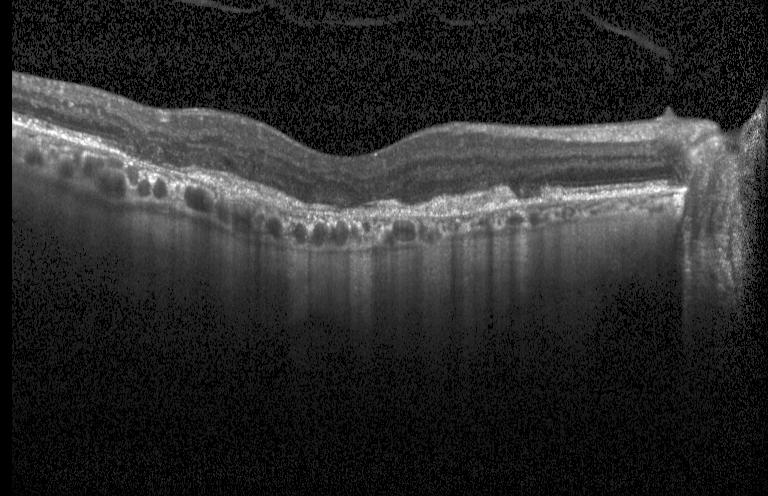 Diagnosis: choroidal neovascularization.